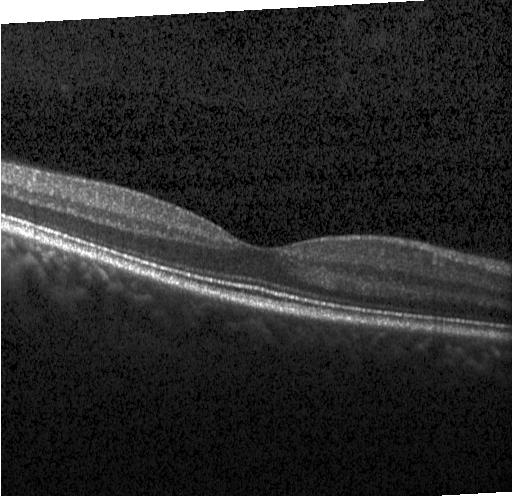

Heidelberg Spectralis OCT system, SD-OCT, OCT B-scan
The scan shows no CNV, DME, or drusen.